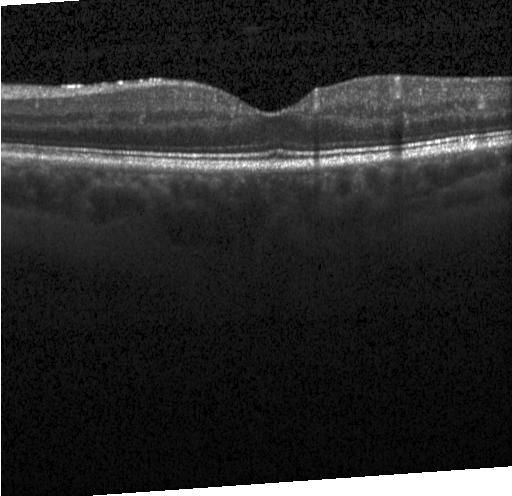 Optical coherence tomography B-scan. OCT finding: no evidence of choroidal neovascularization, diabetic macular edema, or drusen.